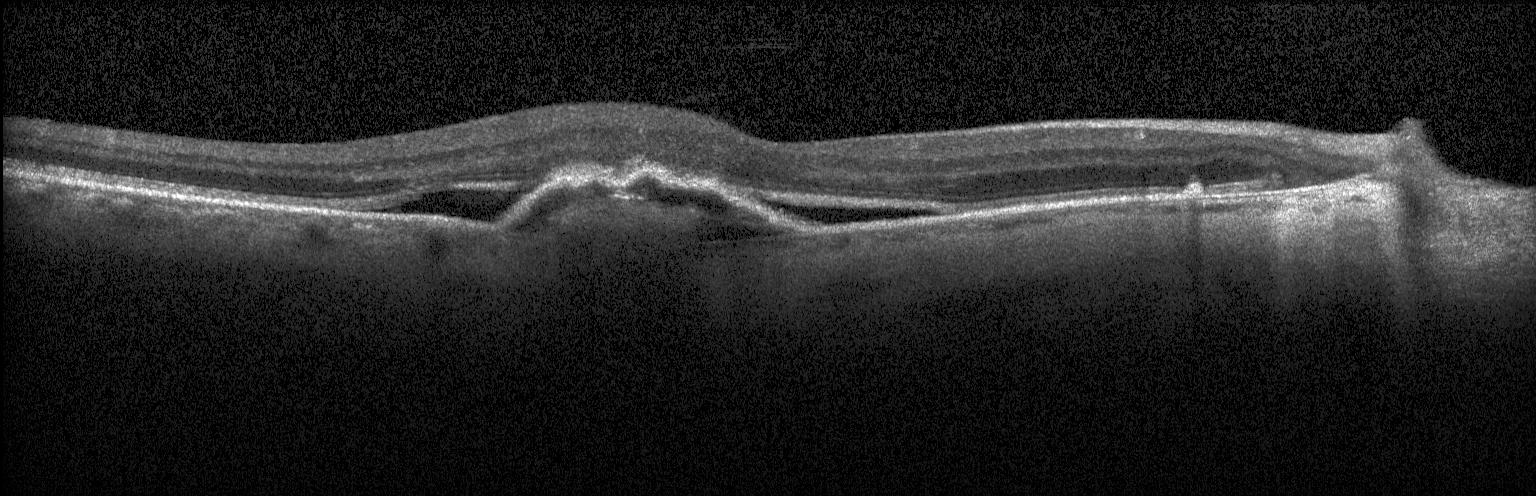

Heidelberg Spectralis; OCT line scan — Dx: CNV.